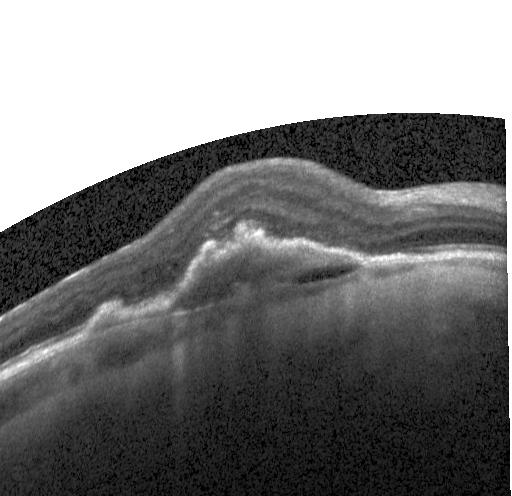 This B-scan demonstrates a choroidal neovascular membrane.